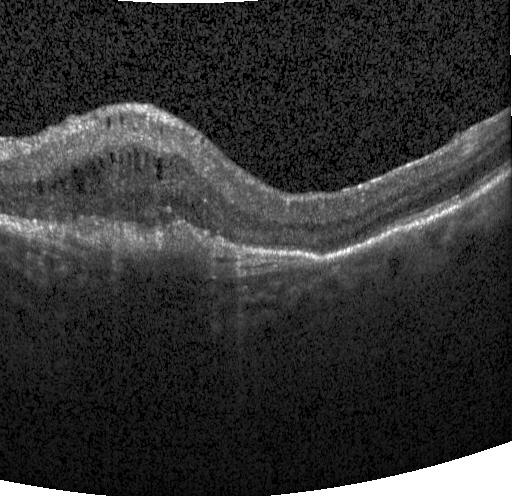

This B-scan demonstrates choroidal neovascularization (CNV).